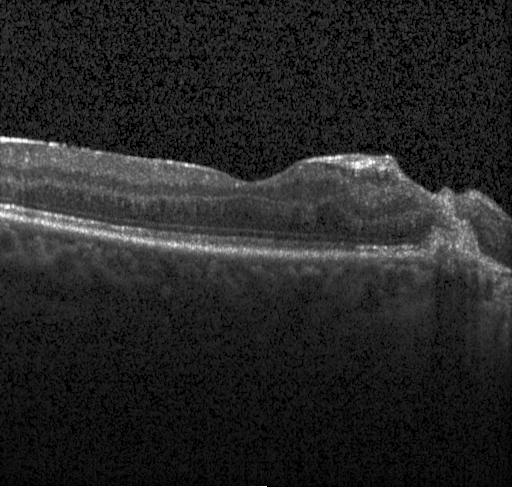 Macular OCT demonstrating a choroidal neovascular membrane.